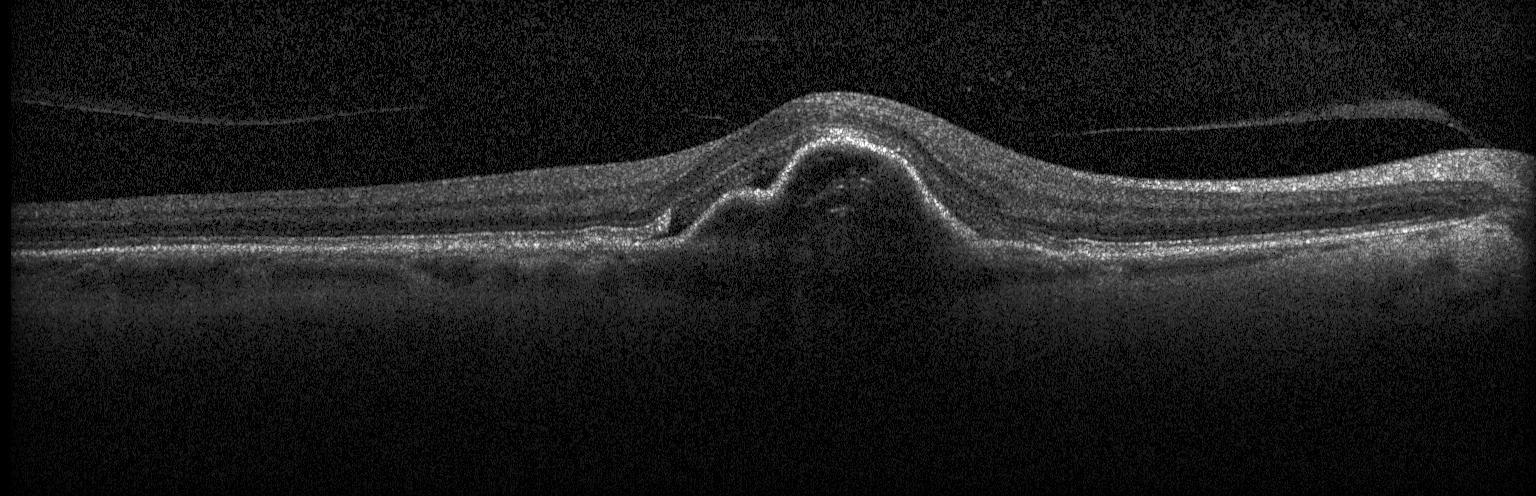
Optical coherence tomography scan. This B-scan demonstrates a choroidal neovascular membrane.